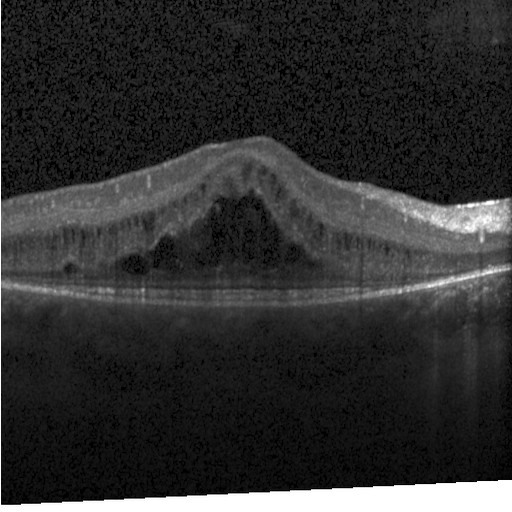

Macular OCT: diabetic macular edema (DME).